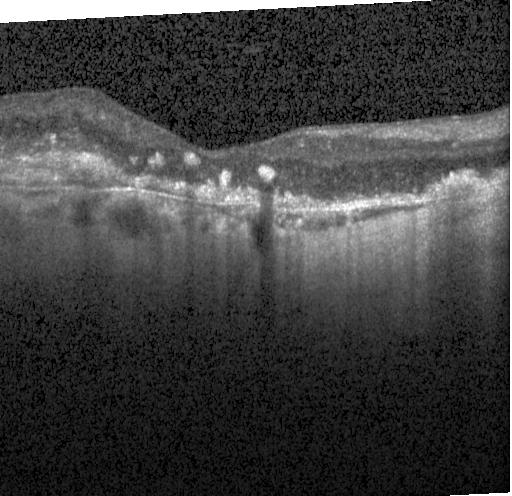

Optical coherence tomography scan · spectral-domain optical coherence tomography · acquired on a Heidelberg Spectralis. Assessment: choroidal neovascularization.